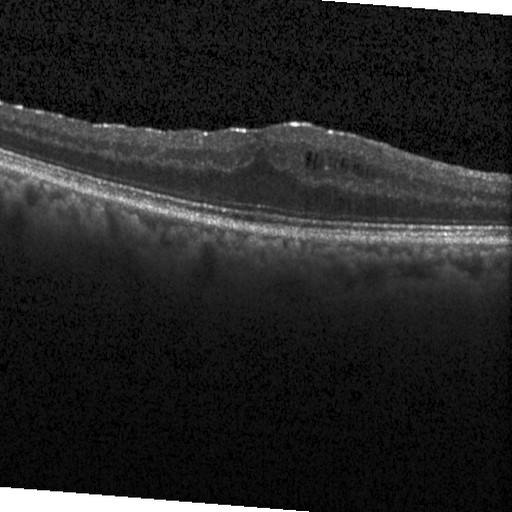
OCT B-scan. Centered on the fovea. Spectral-domain optical coherence tomography. Heidelberg Spectralis OCT system
Impression: DME.